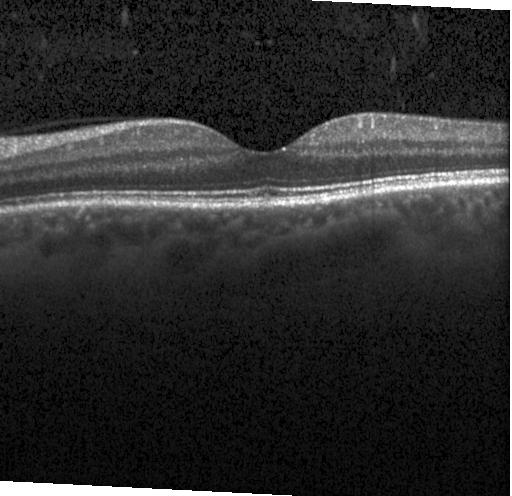

OCT B-scan.
Impression: no CNV, DME, or drusen.